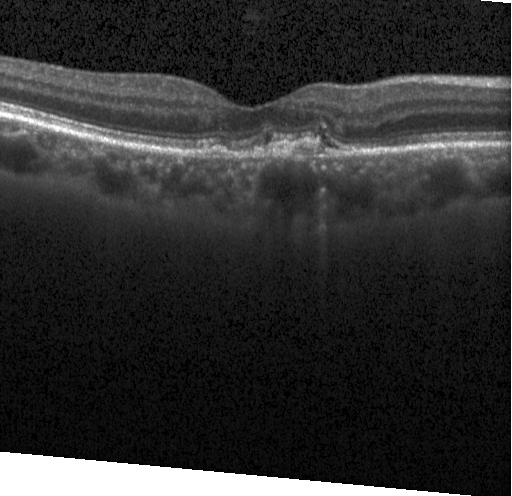 Impression: a choroidal neovascular membrane.